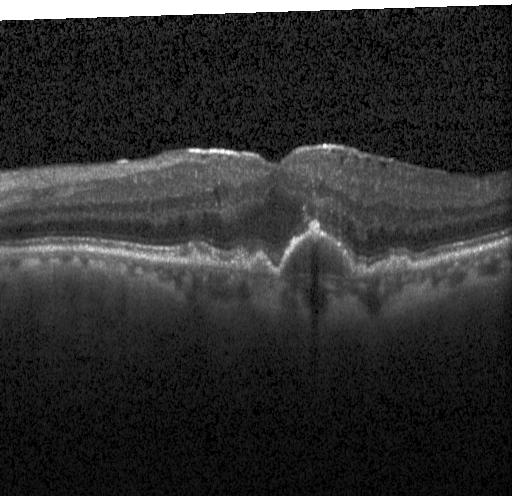
OCT B-scan showing choroidal neovascularization (CNV).